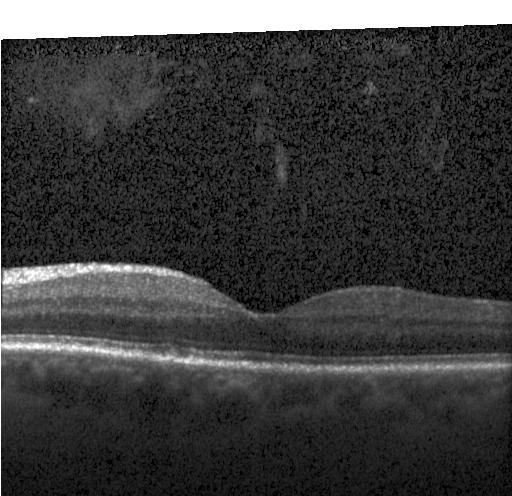

Retinal OCT cross-section; Heidelberg Spectralis OCT system
Diagnosis: no choroidal neovascularization, diabetic macular edema, or drusen.